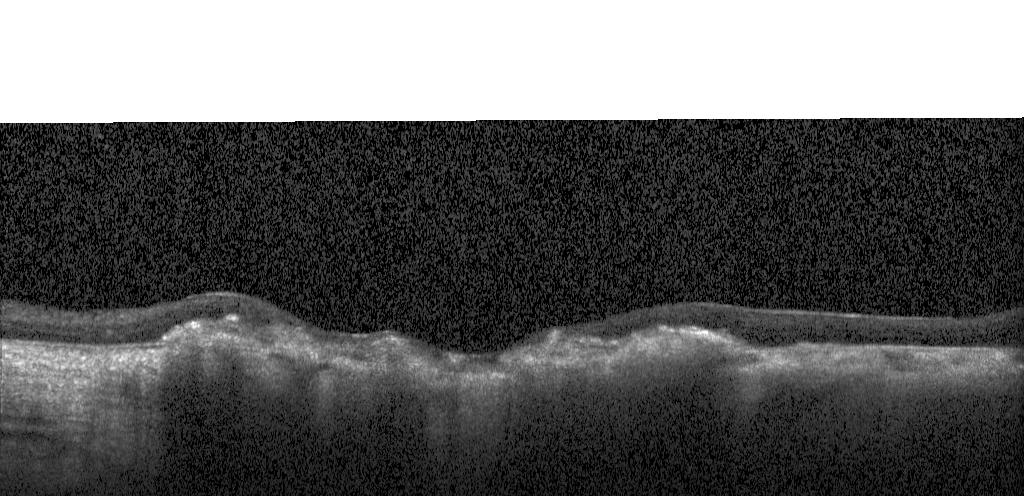
OCT line scan, spectral-domain OCT, instrument: Heidelberg Spectralis, centered on the fovea
Dx: a choroidal neovascular membrane.